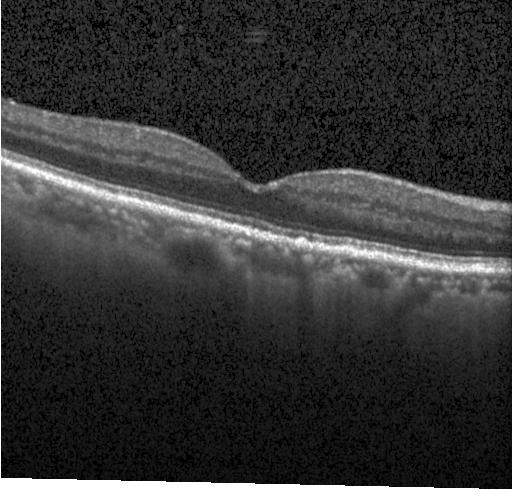 Optical coherence tomography B-scan. Spectral-domain optical coherence tomography.
Finding: no evidence of CNV, DME, or drusen.